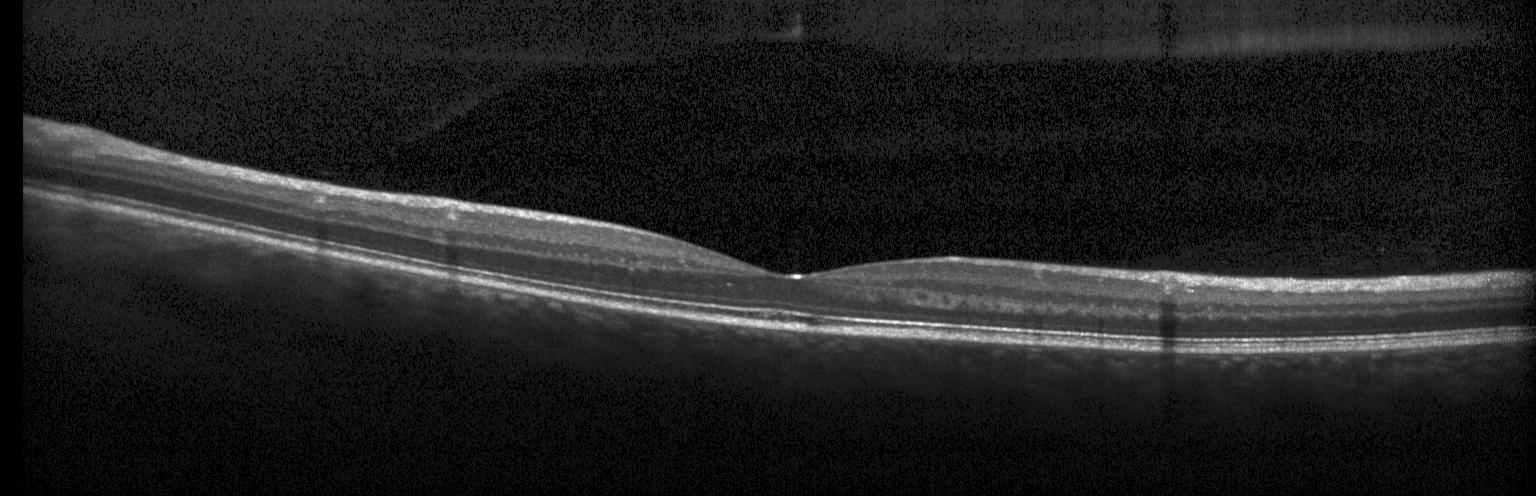

Heidelberg Spectralis OCT system, SD-OCT, retinal OCT B-scan. No evidence of choroidal neovascularization, diabetic macular edema, or drusen.